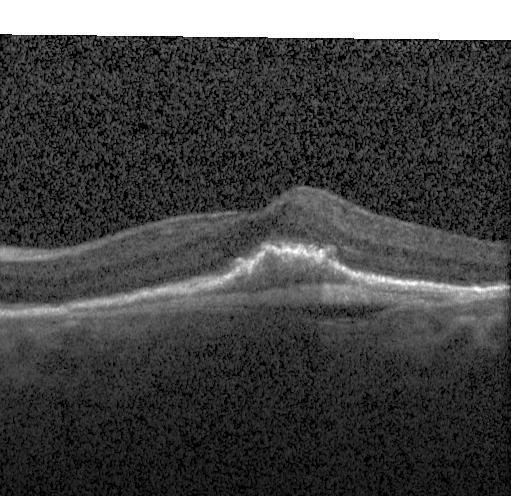

Heidelberg Spectralis; optical coherence tomography scan — Finding: CNV.